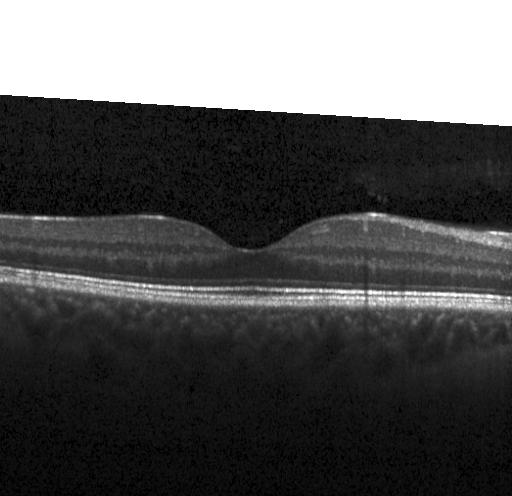
Assessment: neither choroidal neovascularization, diabetic macular edema, nor drusen.